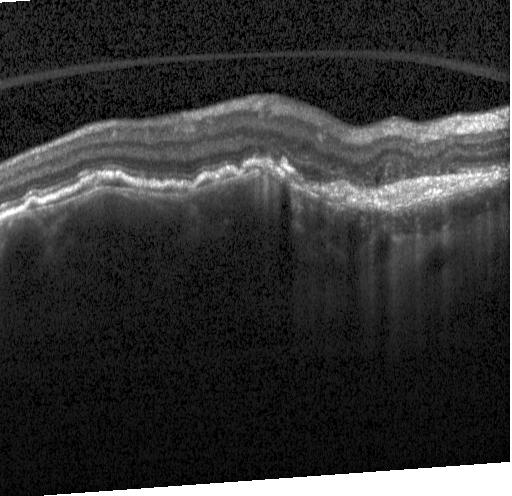 Instrument: Heidelberg Spectralis, spectral-domain optical coherence tomography, optical coherence tomography scan, horizontal scan through the fovea. The scan shows choroidal neovascularization (CNV).